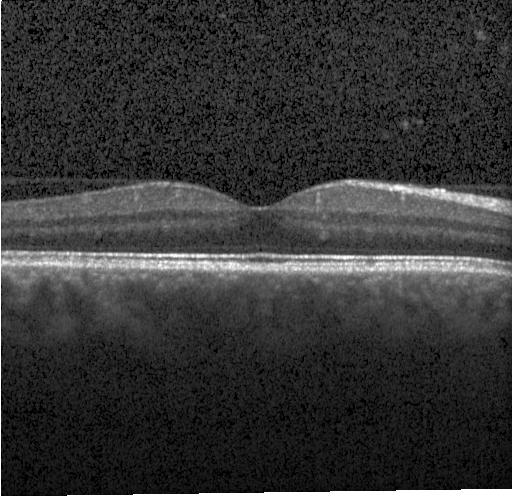 OCT line scan
No choroidal neovascularization, no diabetic macular edema, and no drusen.